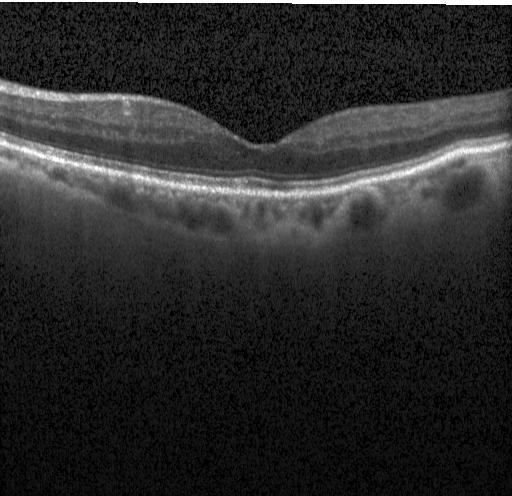 Macular OCT demonstrating neither choroidal neovascularization, diabetic macular edema, nor drusen.